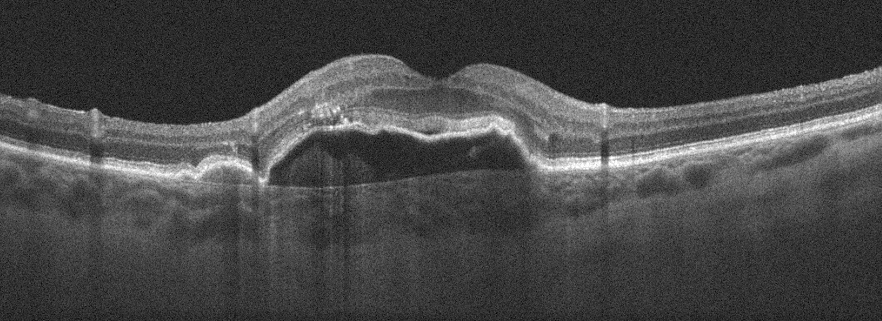

Spectral-domain OCT B-scan: age-related macular degeneration.